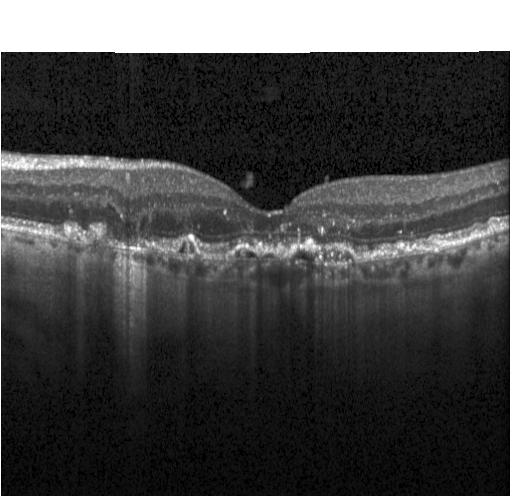 Macular OCT demonstrating choroidal neovascularization (CNV).